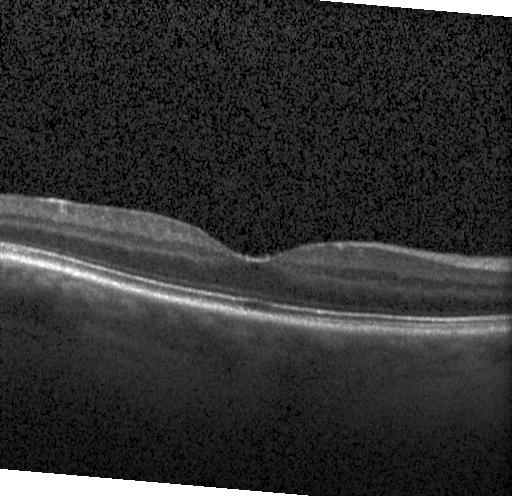

Retinal OCT cross-section. Acquired on a Heidelberg Spectralis. Diagnosis: no evidence of choroidal neovascularization, diabetic macular edema, or drusen.